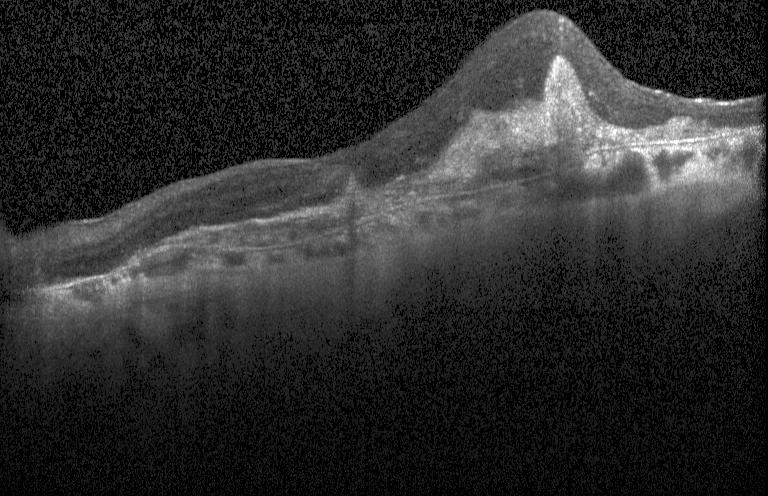
OCT B-scan — A choroidal neovascular membrane.